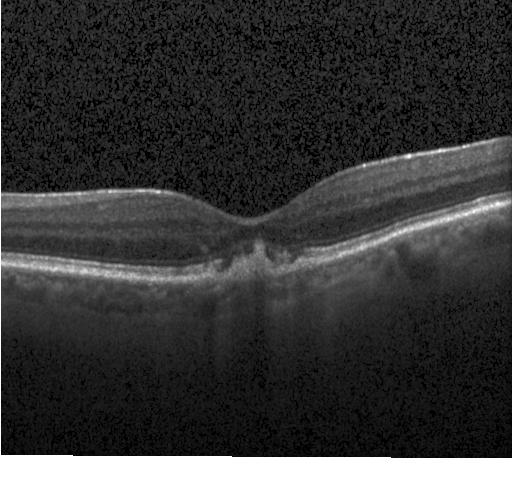

Spectral-domain optical coherence tomography. Heidelberg Spectralis OCT system. Optical coherence tomography scan. Macular scan. This B-scan demonstrates a choroidal neovascular membrane.